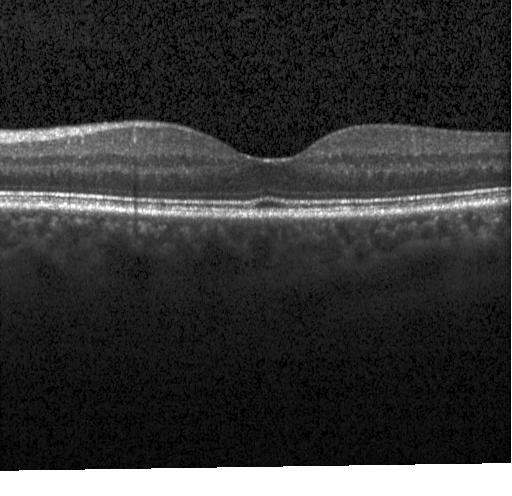

Optical coherence tomography scan, SD-OCT, centered on the fovea, acquired on a Heidelberg Spectralis
Finding: neither CNV, DME, nor drusen.